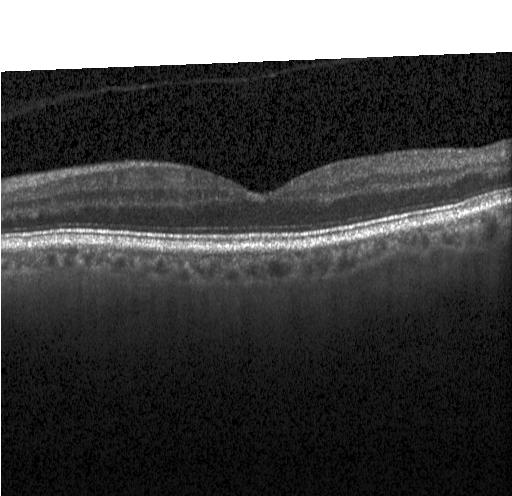
Retinal OCT cross-section
Impression: no CNV, DME, or drusen.